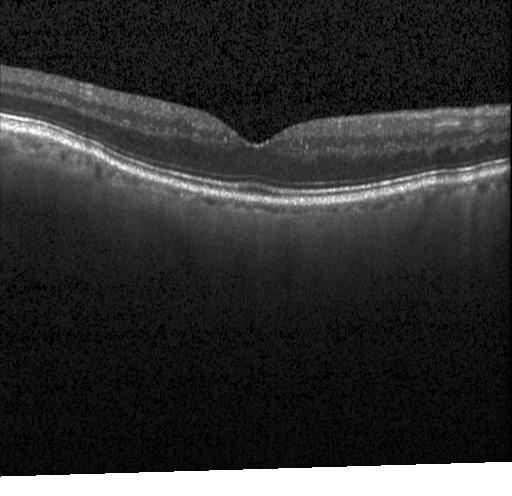 OCT B-scan showing no choroidal neovascularization, no diabetic macular edema, and no drusen.